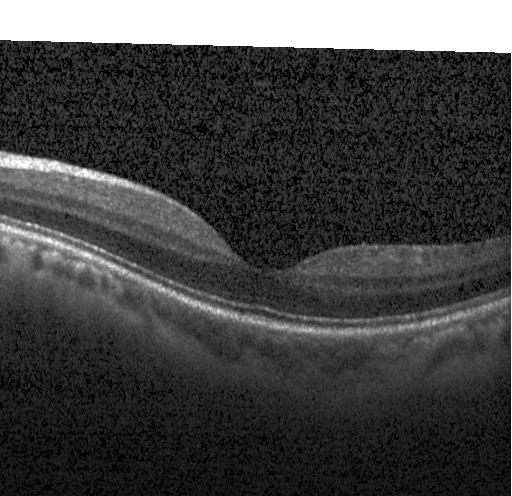

OCT scan showing no CNV, DME, or drusen.